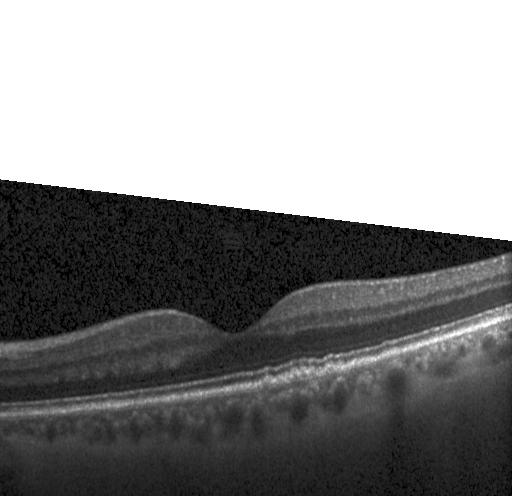
Optical coherence tomography B-scan. Heidelberg Spectralis.
Diagnosis: drusen.